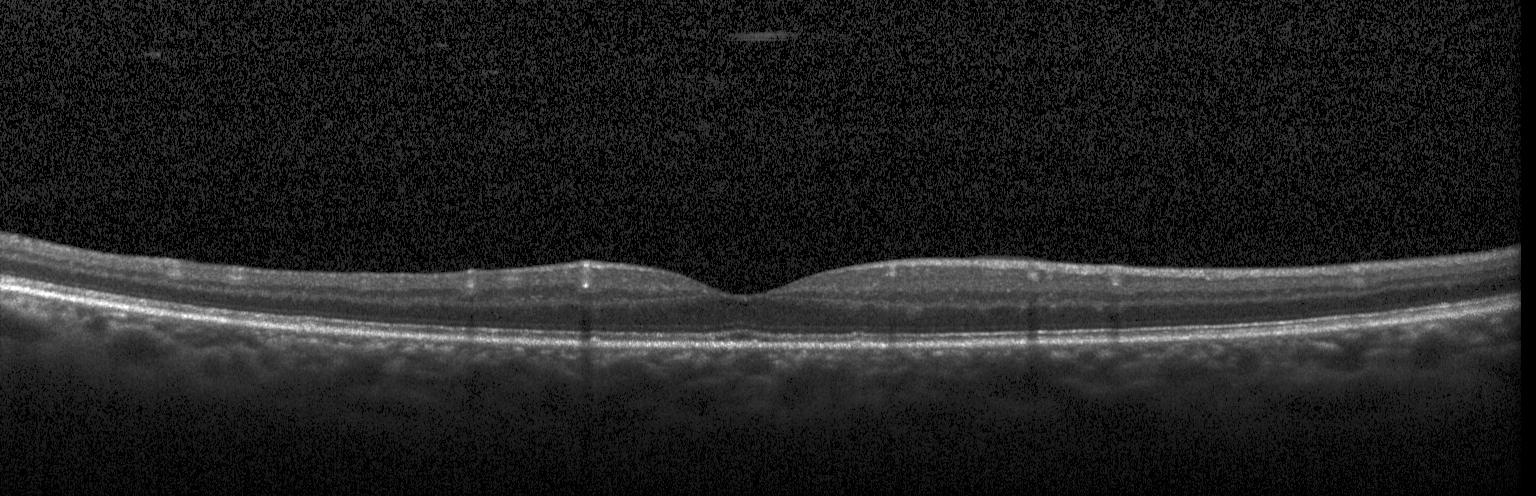

Spectral-domain OCT. Through the macula. OCT line scan. Finding: no choroidal neovascularization, no diabetic macular edema, and no drusen.